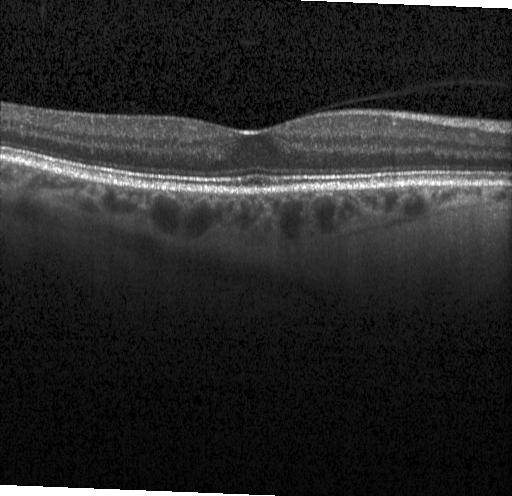
SD-OCT. Optical coherence tomography B-scan.
Finding: no evidence of choroidal neovascularization, diabetic macular edema, or drusen.